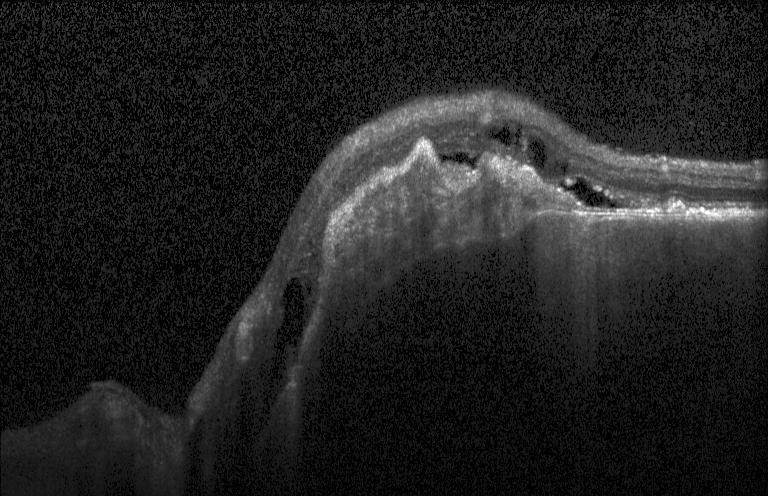 Dx: choroidal neovascularization.